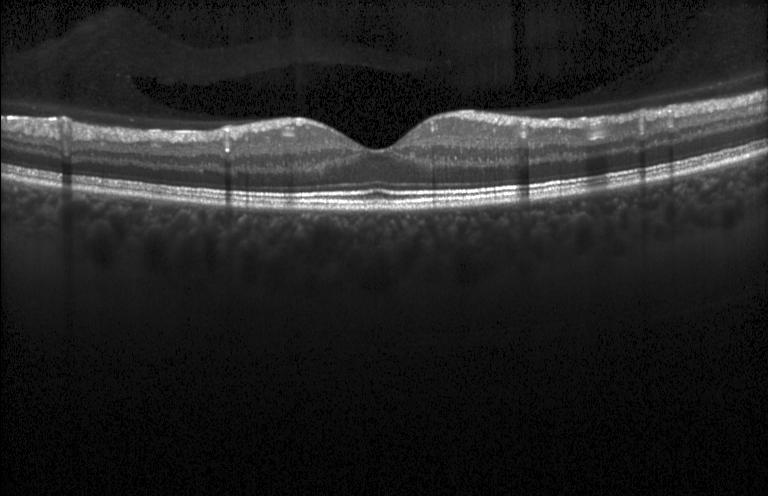
OCT B-scan; Heidelberg Spectralis.
This B-scan demonstrates no evidence of CNV, DME, or drusen.